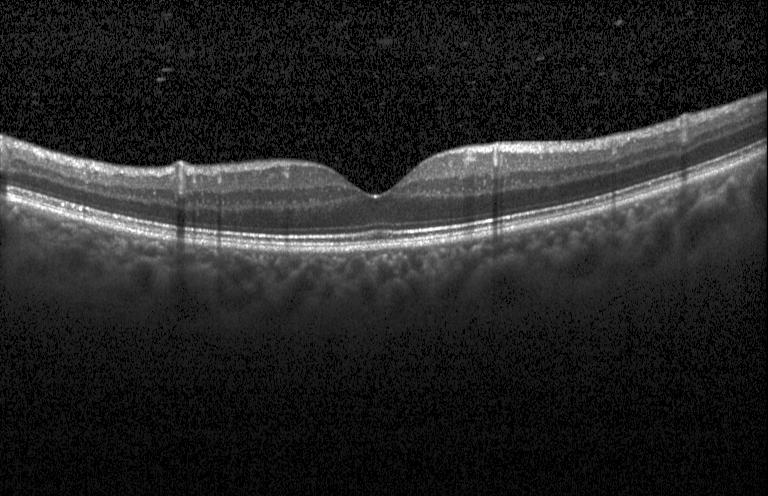

Heidelberg Spectralis OCT system. OCT B-scan. Through the macula.
The scan shows no evidence of CNV, DME, or drusen.